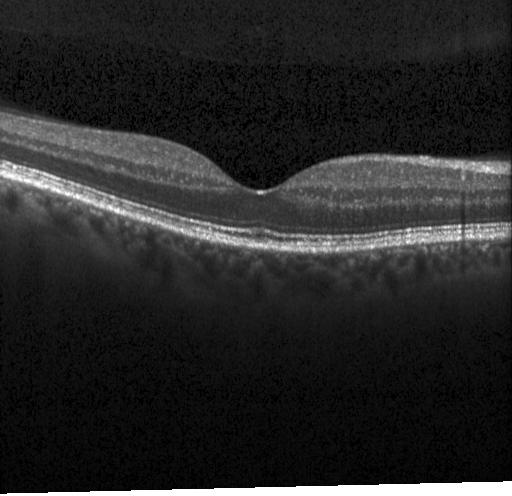

Spectral-domain OCT B-scan: no choroidal neovascularization, diabetic macular edema, or drusen.